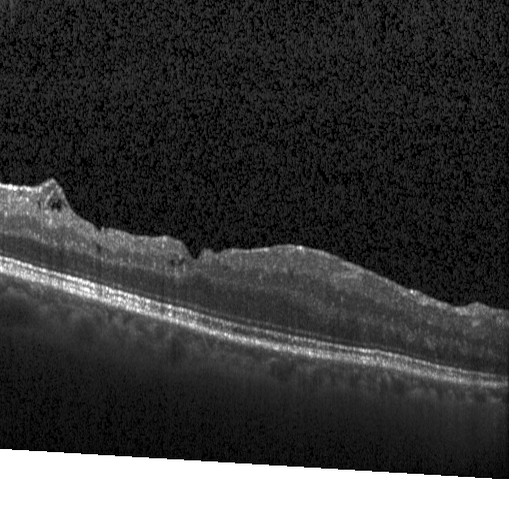 Finding: diabetic macular edema.